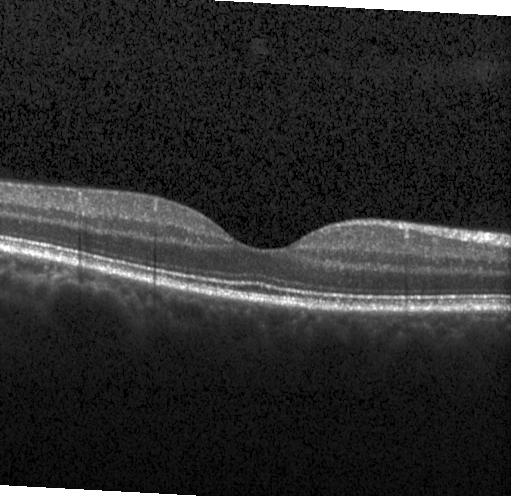

OCT line scan.
The scan shows no choroidal neovascularization, diabetic macular edema, or drusen.